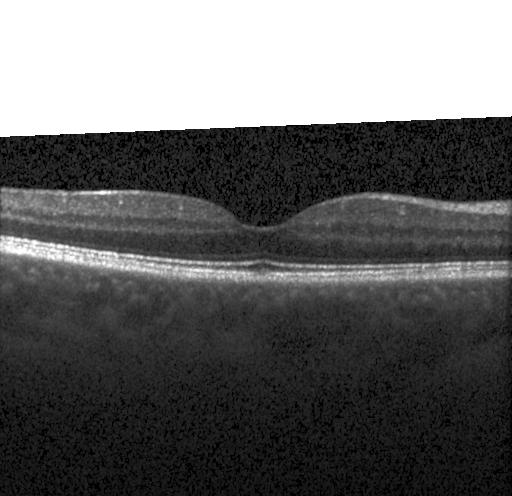

Retinal OCT B-scan · fovea-centered.
Diagnosis: no choroidal neovascularization, diabetic macular edema, or drusen.